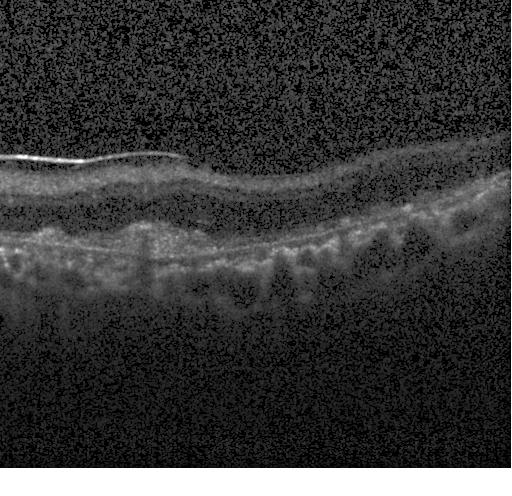

Optical coherence tomography scan — This B-scan demonstrates a choroidal neovascular membrane.